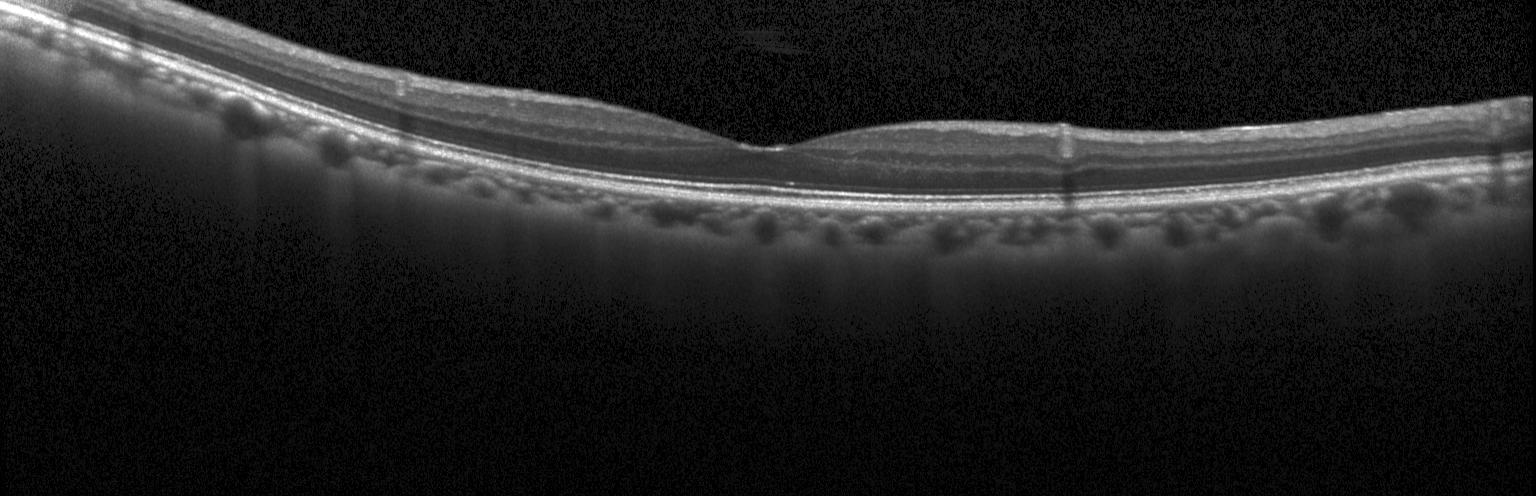
Dx: no evidence of choroidal neovascularization, diabetic macular edema, or drusen.